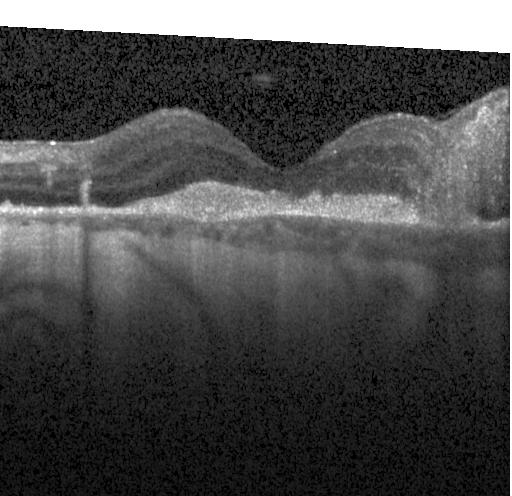

Assessment: a choroidal neovascular membrane.